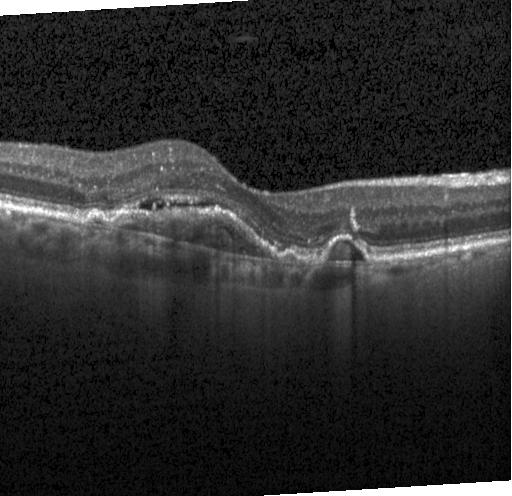
Retinal OCT B-scan
Diagnosis: a choroidal neovascular membrane.